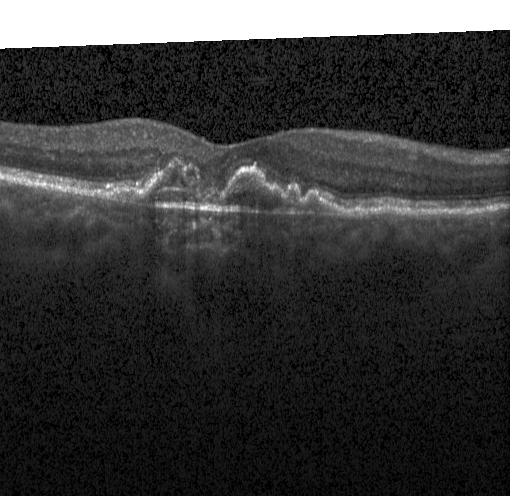 A choroidal neovascular membrane.